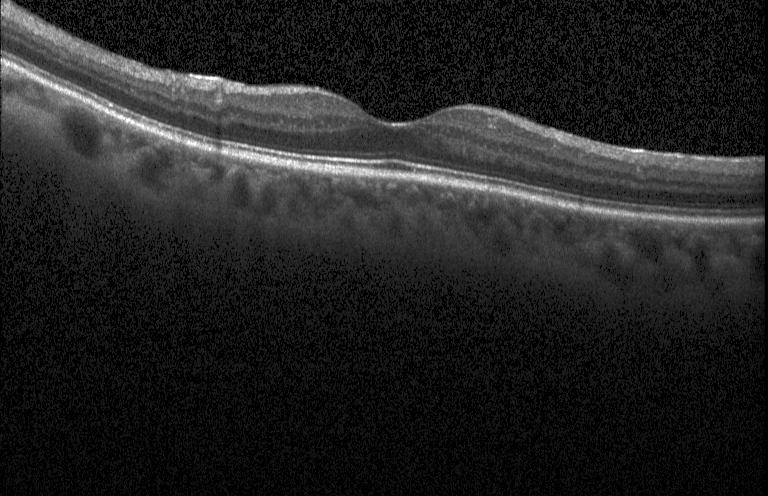
Diagnosis: no CNV, no DME, and no drusen.